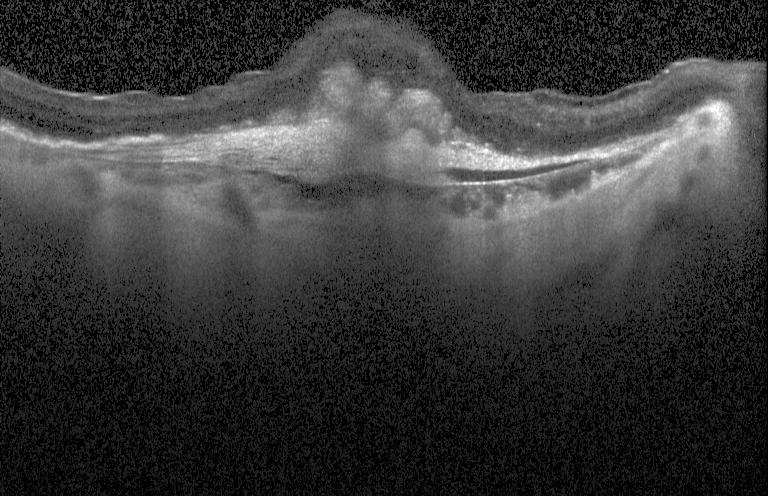
Macular OCT demonstrating choroidal neovascularization (CNV).